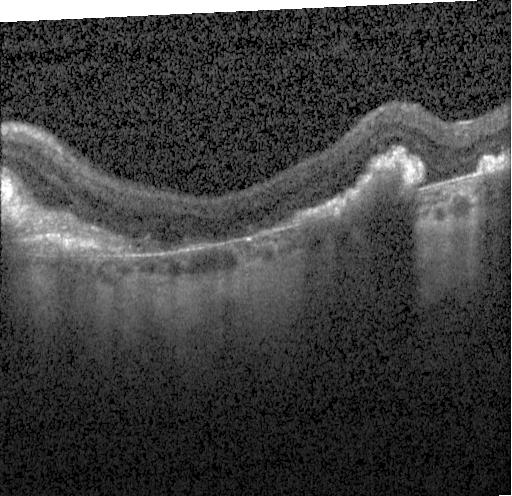
Spectral-domain OCT B-scan: choroidal neovascularization.